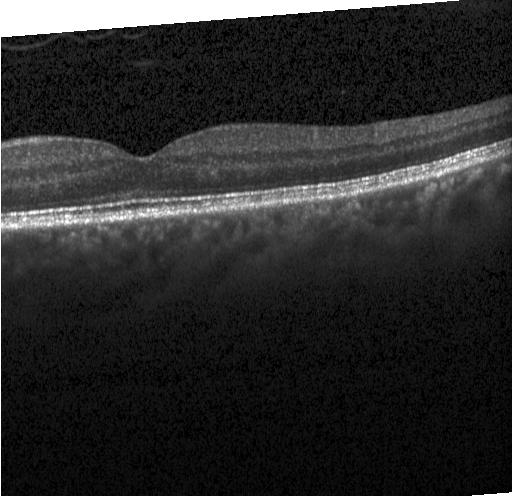 Macular OCT demonstrating no CNV, no DME, and no drusen.